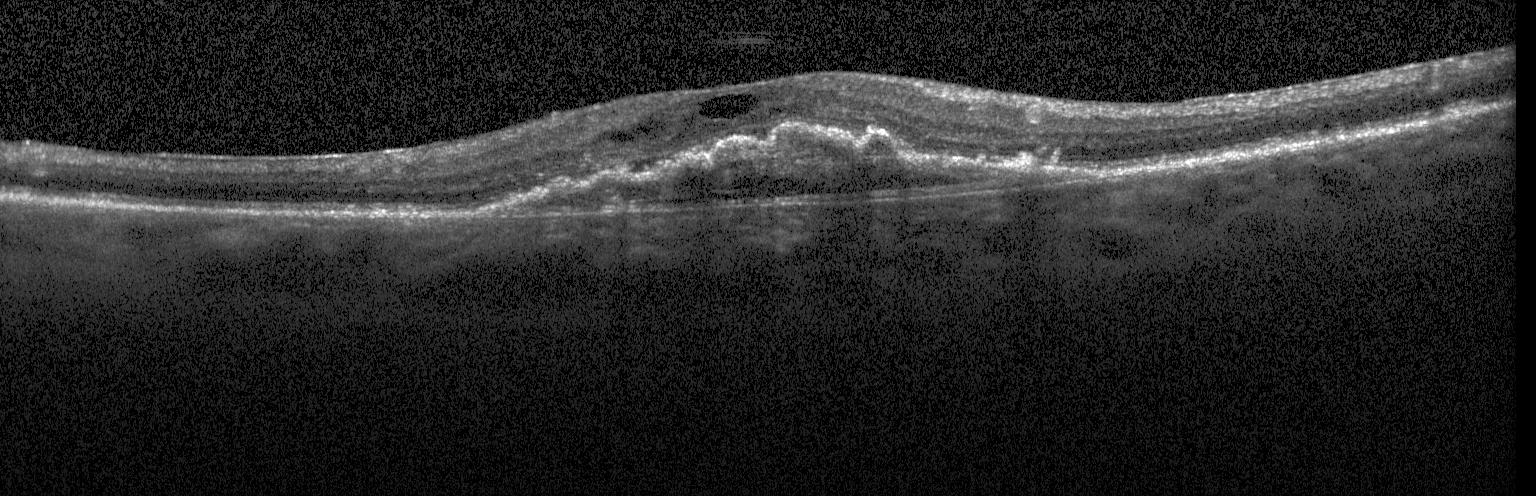

Heidelberg Spectralis OCT system · optical coherence tomography scan
Finding: a choroidal neovascular membrane.